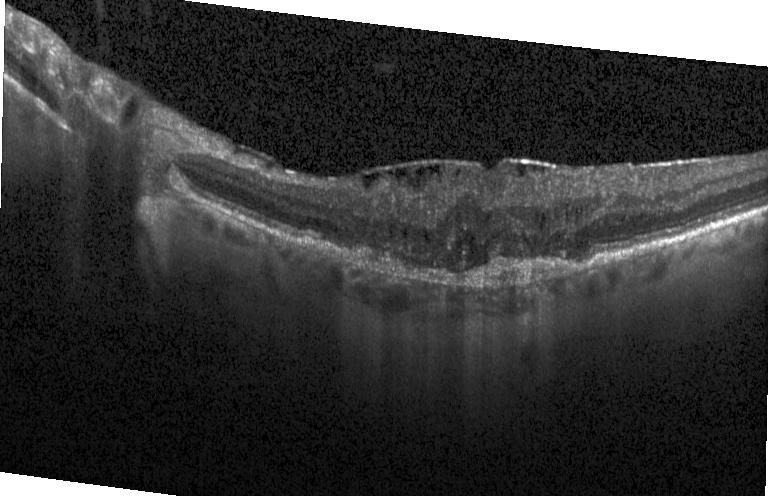 Impression: choroidal neovascularization.